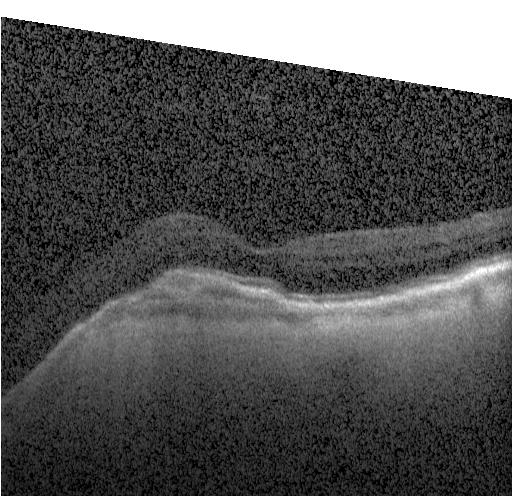
Horizontal scan through the fovea. Retinal OCT cross-section. Acquired on a Heidelberg Spectralis. SD-OCT.
Impression: choroidal neovascularization.